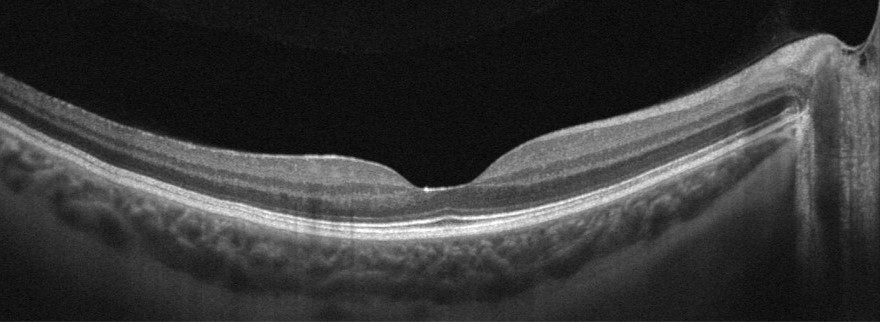 OCT line scan. The scan shows no evidence of AMD, DME, ERM, RAO, RVO, or VID.